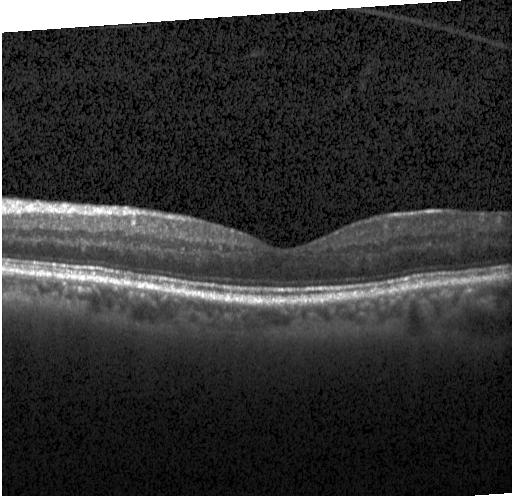
Optical coherence tomography scan · through the macula · spectral-domain OCT · acquired on a Heidelberg Spectralis — Finding: no CNV, DME, or drusen.